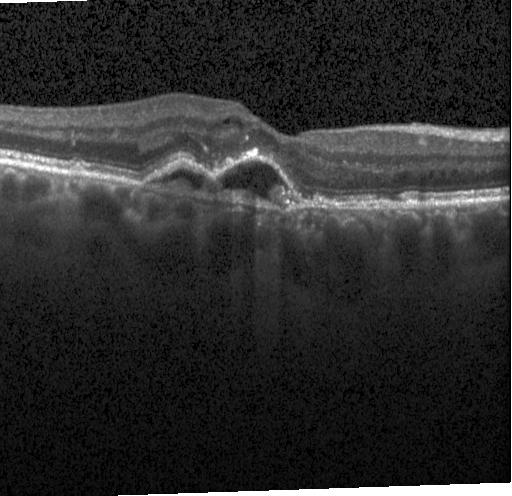 Spectral-domain optical coherence tomography; retinal OCT cross-section — OCT finding: a choroidal neovascular membrane.